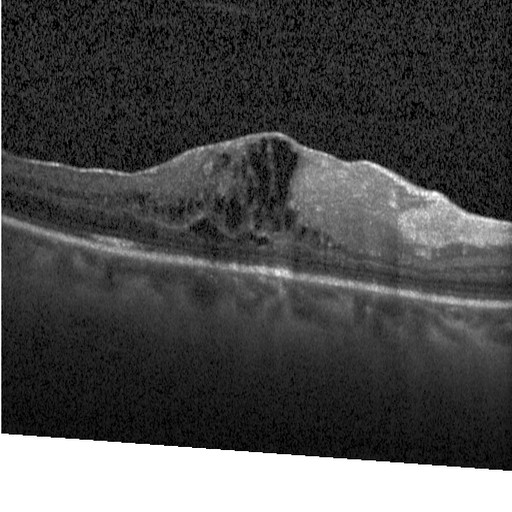

Retinal OCT cross-section. Spectral-domain optical coherence tomography. Heidelberg Spectralis OCT system. Finding: DME.